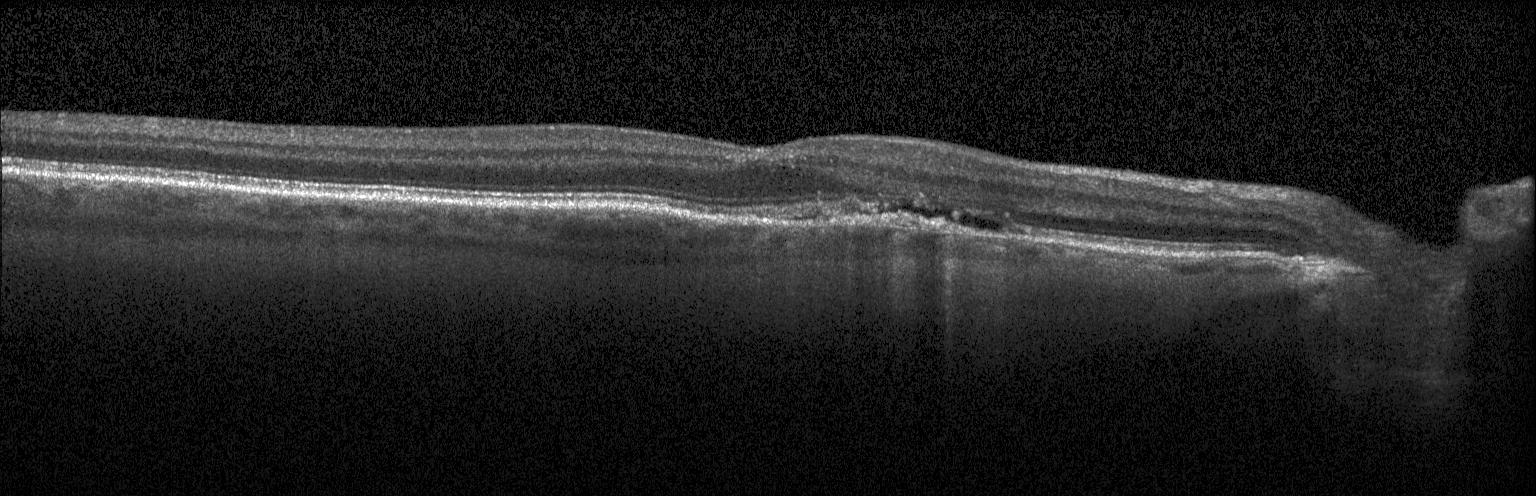 Optical coherence tomography B-scan, acquired on a Heidelberg Spectralis, SD-OCT, centered on the fovea
This B-scan demonstrates a choroidal neovascular membrane.